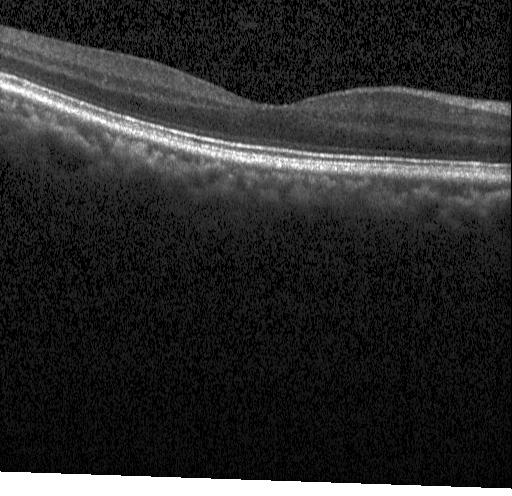 Retinal OCT cross-section · spectral-domain optical coherence tomography. No choroidal neovascularization, no diabetic macular edema, and no drusen.